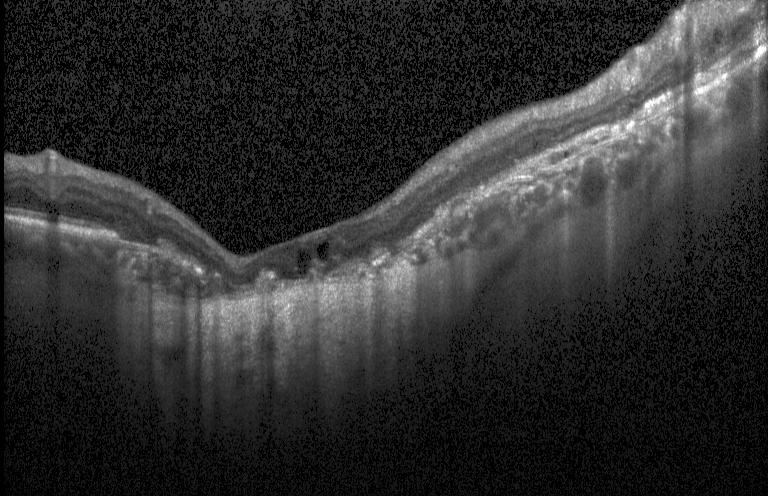
Optical coherence tomography B-scan. Diagnosis: CNV.